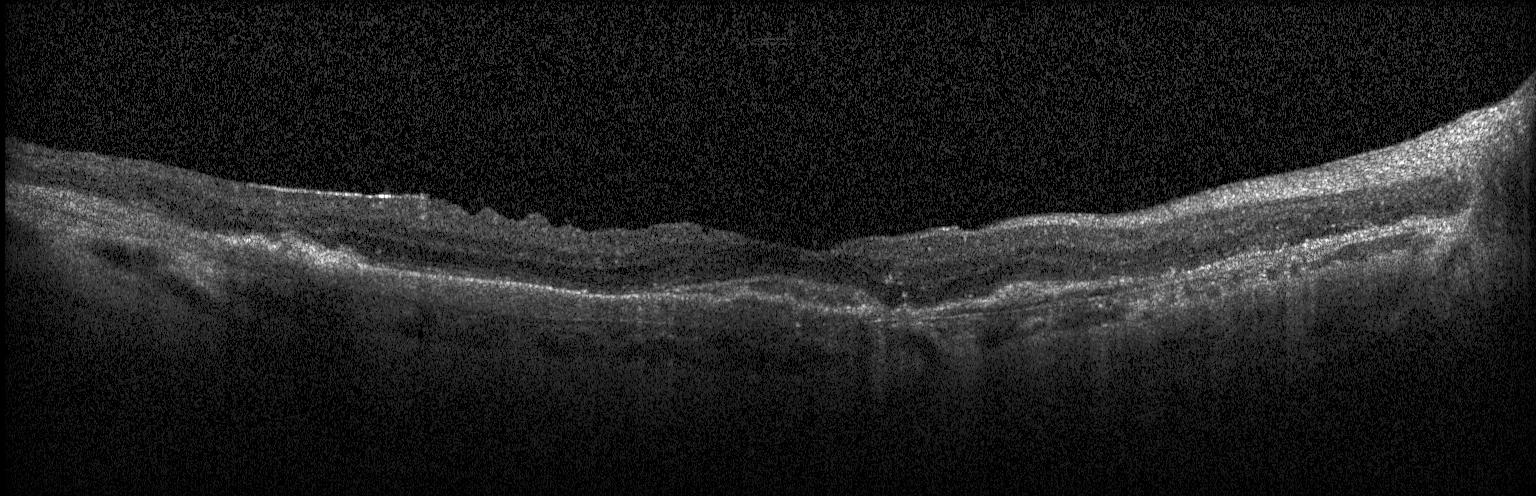 Retinal OCT B-scan, instrument: Heidelberg Spectralis
This B-scan demonstrates a choroidal neovascular membrane.